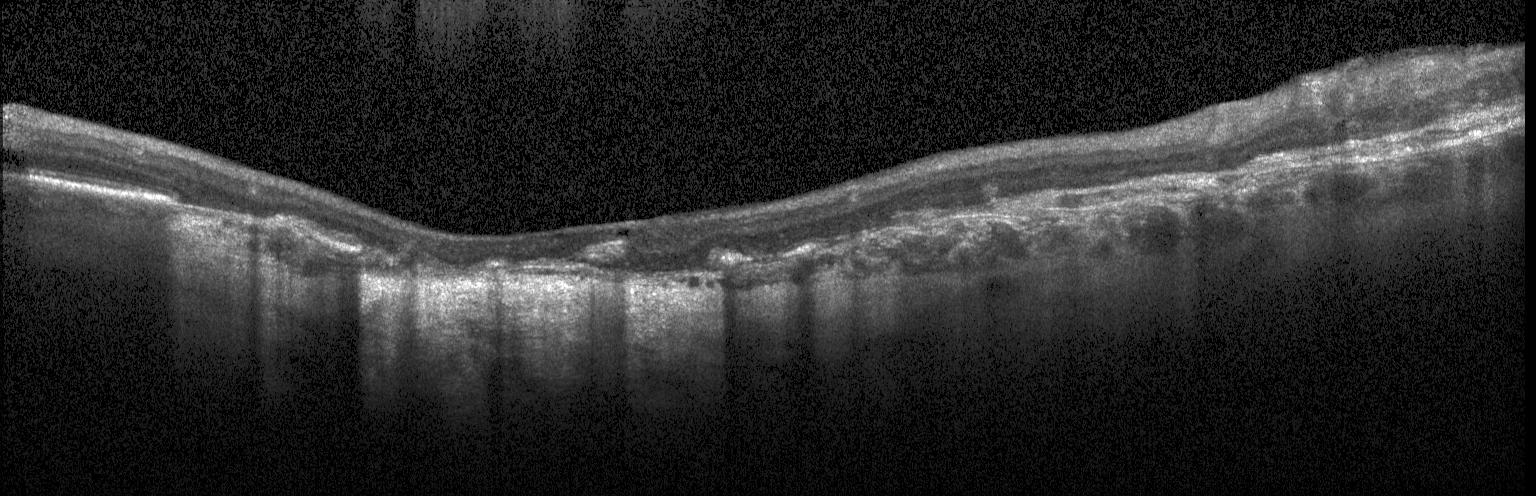
Retinal OCT B-scan. Spectral-domain OCT. Heidelberg Spectralis — This B-scan demonstrates a choroidal neovascular membrane.